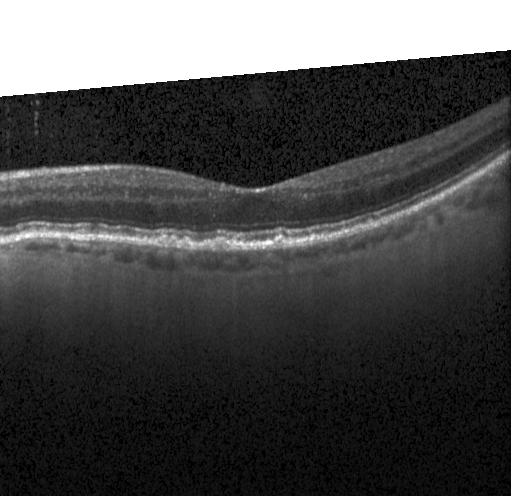

The scan shows multiple drusen.